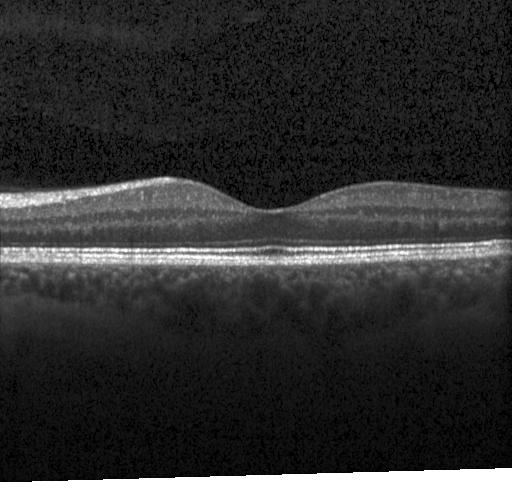 Diagnosis: no choroidal neovascularization, diabetic macular edema, or drusen.